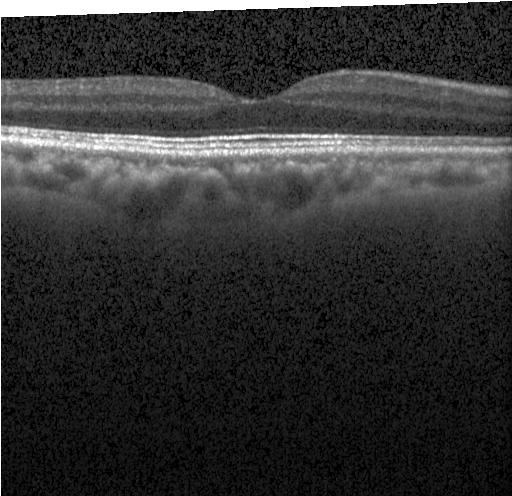
Instrument: Heidelberg Spectralis. OCT B-scan. Centered on the fovea
Impression: neither choroidal neovascularization, diabetic macular edema, nor drusen.